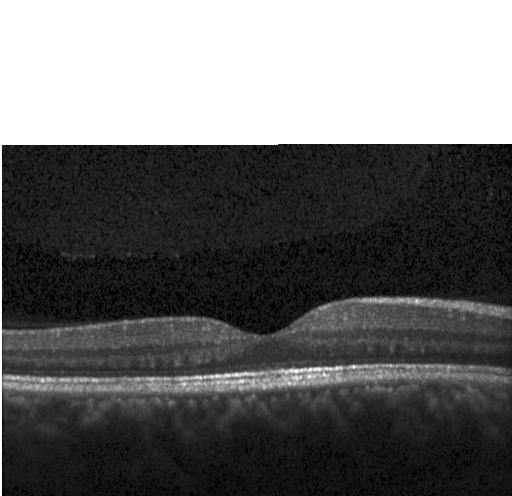
Spectral-domain optical coherence tomography; retinal OCT B-scan; acquired on a Heidelberg Spectralis
Assessment: no choroidal neovascularization, diabetic macular edema, or drusen.